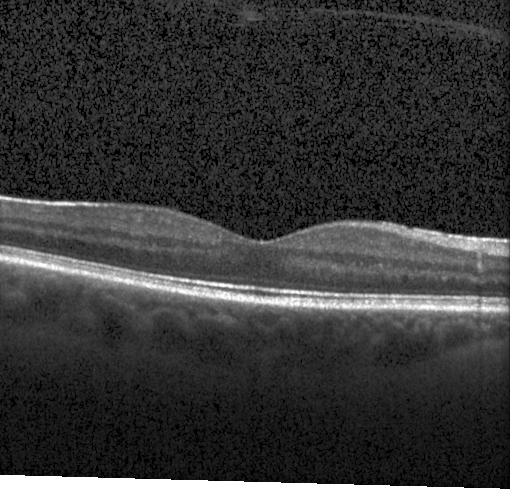 Finding: no choroidal neovascularization, no diabetic macular edema, and no drusen.